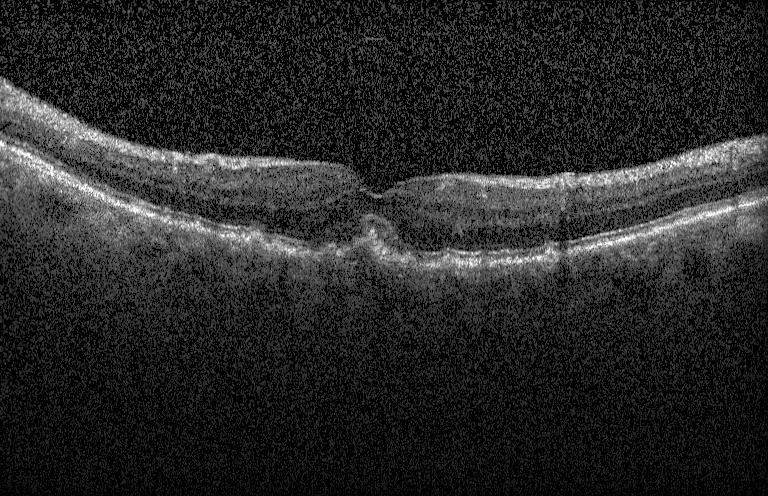

Finding: CNV.